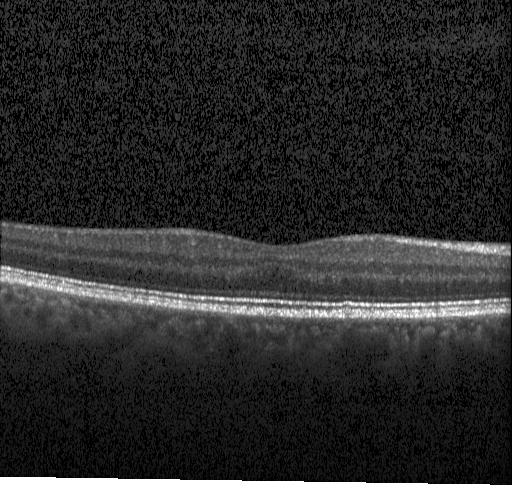
Acquired on a Heidelberg Spectralis; retinal OCT B-scan; macular scan; spectral-domain OCT. Diagnosis: no CNV, no DME, and no drusen.